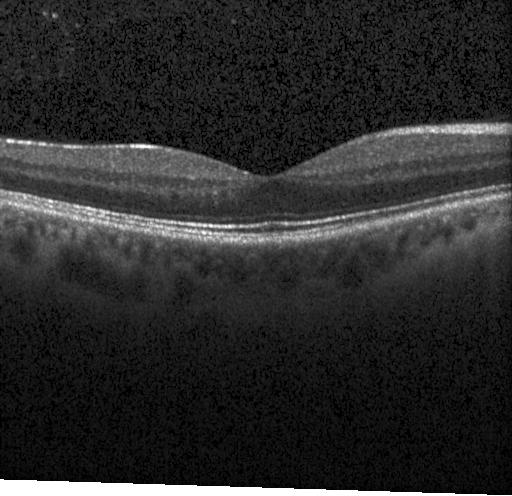
Spectral-domain OCT; OCT line scan; Heidelberg Spectralis OCT system; centered on the fovea — Finding: neither choroidal neovascularization, diabetic macular edema, nor drusen.